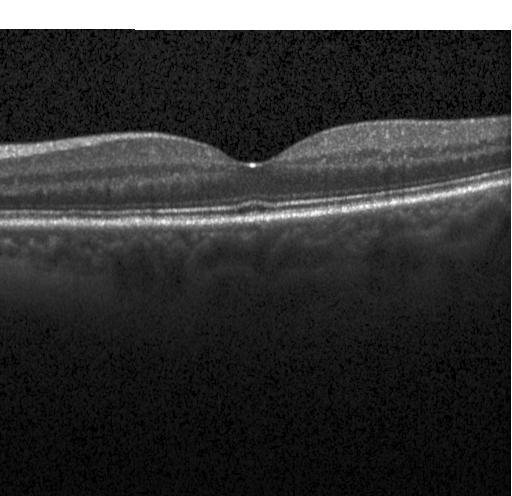
Dx: no choroidal neovascularization, diabetic macular edema, or drusen.